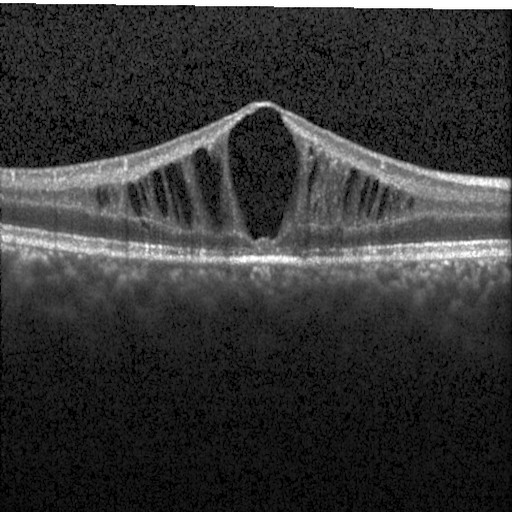

Retinal OCT cross-section showing diabetic macular edema.